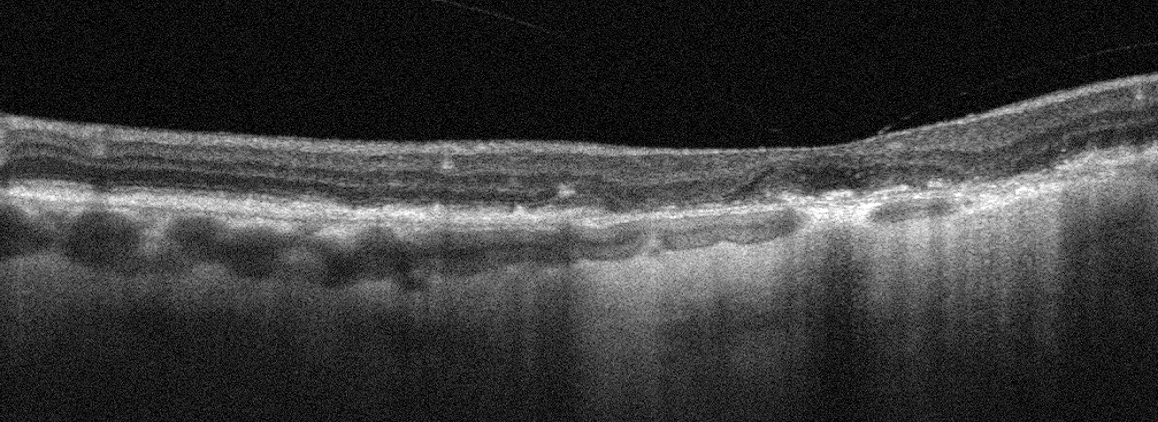 Right eye · OCT B-scan — Finding: age-related macular degeneration (AMD).